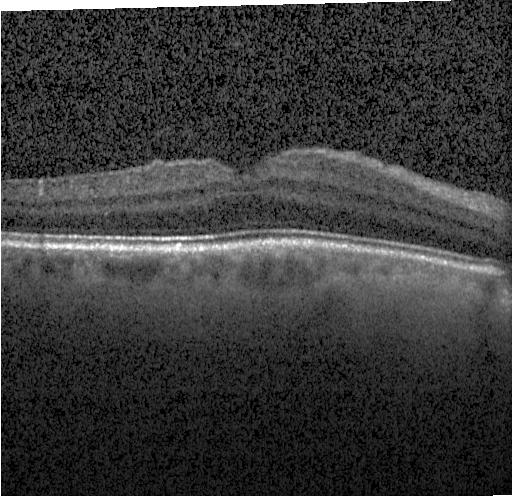

Neither choroidal neovascularization, diabetic macular edema, nor drusen.